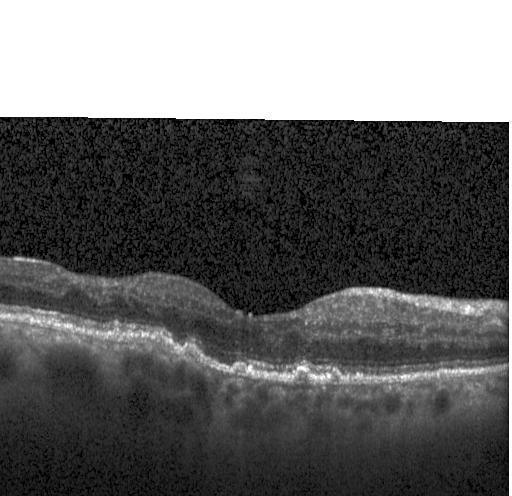 Optical coherence tomography B-scan, Heidelberg Spectralis, SD-OCT, fovea-centered. Drusen.